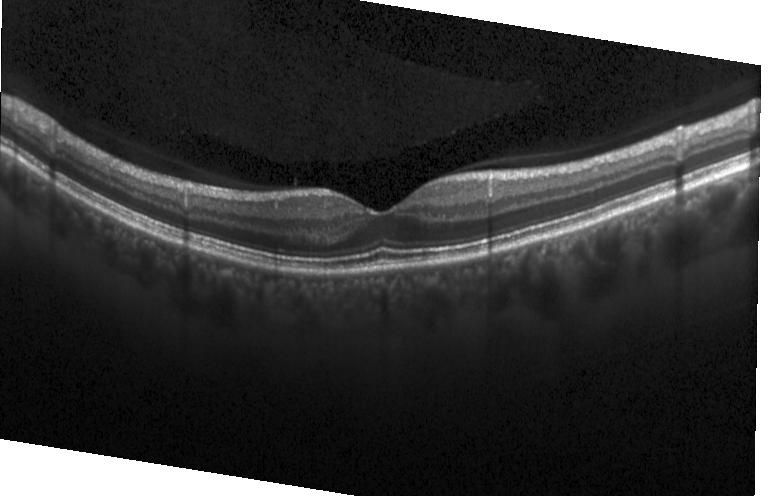

Heidelberg Spectralis; OCT line scan; through the macula; spectral-domain optical coherence tomography.
Diagnosis: no CNV, DME, or drusen.